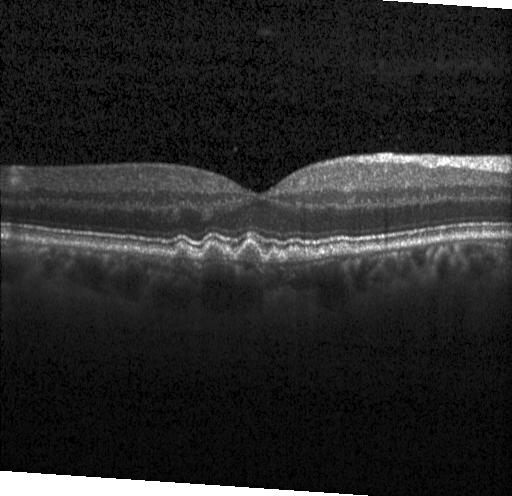

Spectral-domain OCT; Heidelberg Spectralis; through the macula; optical coherence tomography B-scan. OCT finding: drusen.